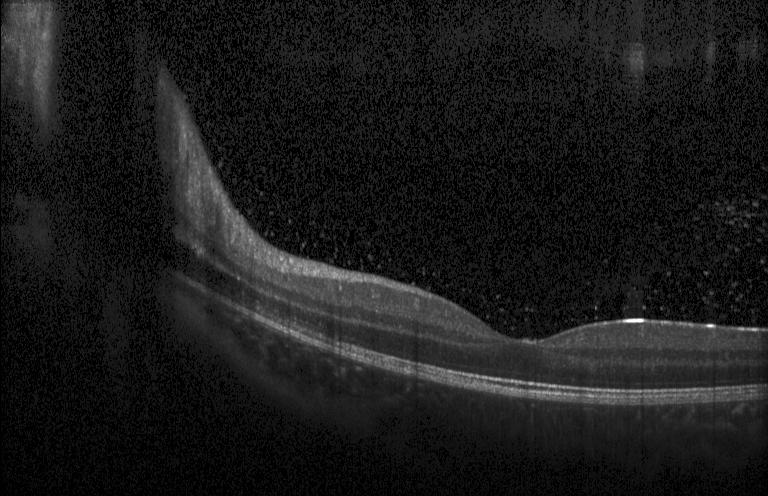
Horizontal scan through the fovea, retinal OCT cross-section — No choroidal neovascularization, no diabetic macular edema, and no drusen.